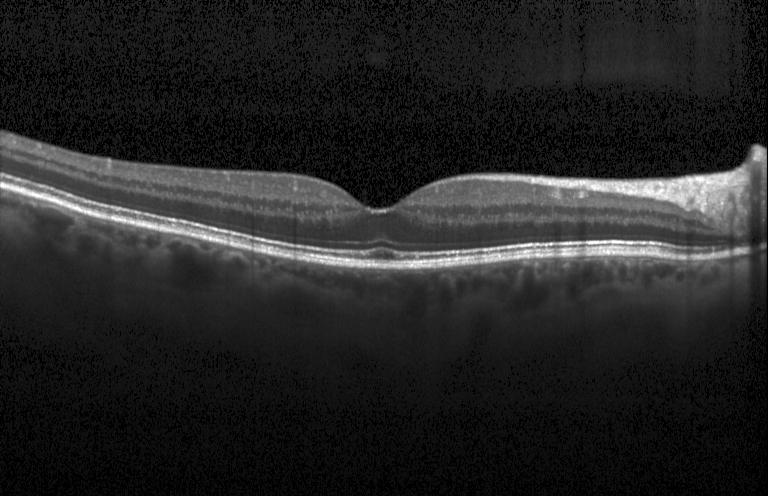 Spectral-domain OCT B-scan: no evidence of choroidal neovascularization, diabetic macular edema, or drusen.